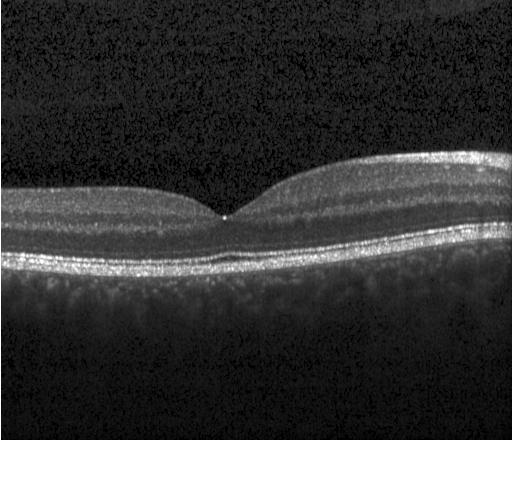
Optical coherence tomography scan — Neither CNV, DME, nor drusen.